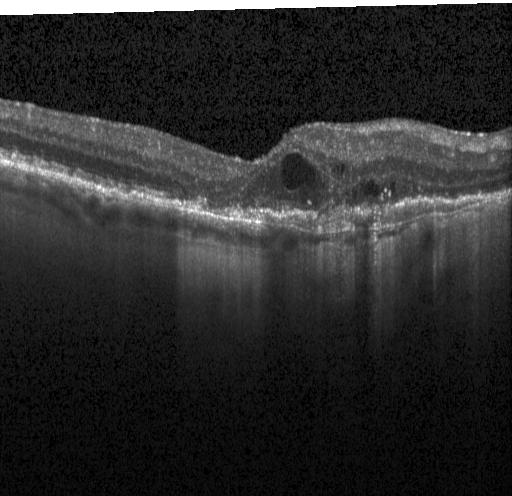

Optical coherence tomography B-scan. Acquired on a Heidelberg Spectralis. Fovea-centered. SD-OCT
A choroidal neovascular membrane.